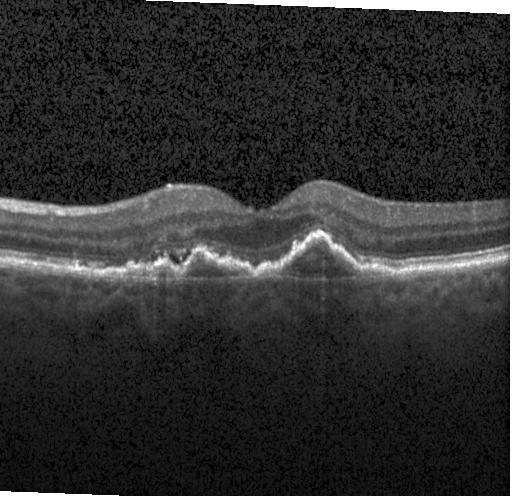
Finding: choroidal neovascularization.